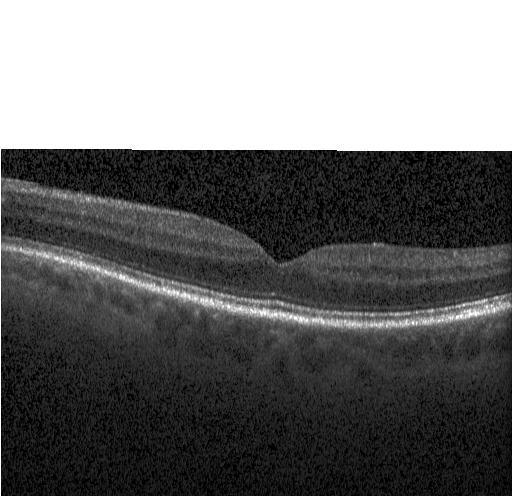

OCT B-scan. Dx: no choroidal neovascularization, diabetic macular edema, or drusen.